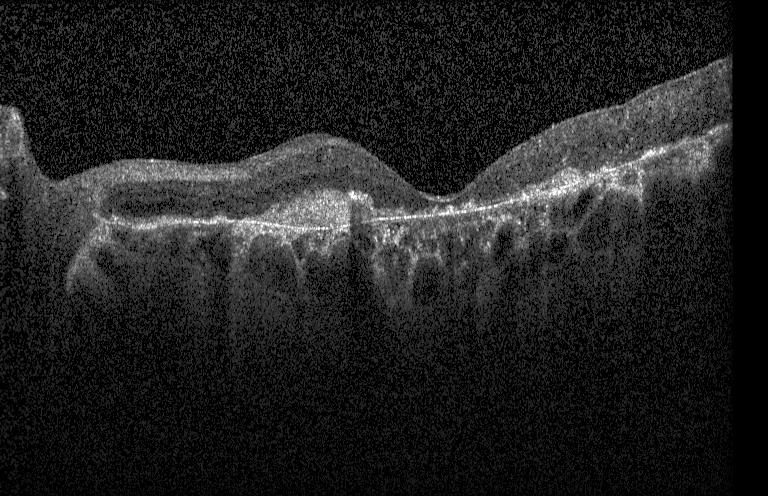
Macular scan; SD-OCT; retinal OCT B-scan
Impression: choroidal neovascularization.